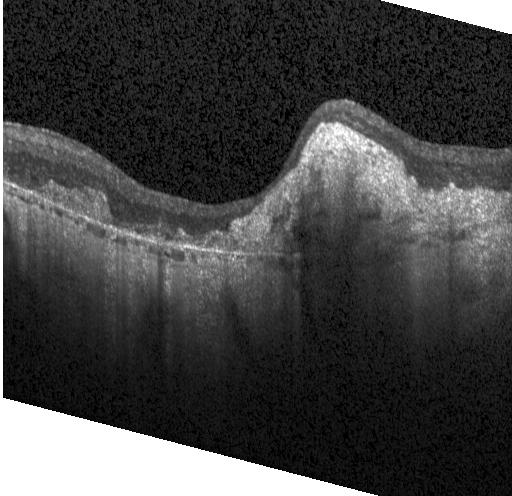

Retinal OCT B-scan; centered on the fovea; SD-OCT.
Dx: a choroidal neovascular membrane.